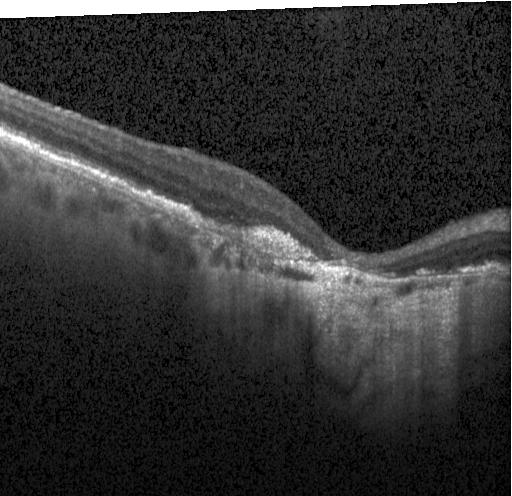
Optical coherence tomography B-scan. Choroidal neovascularization.